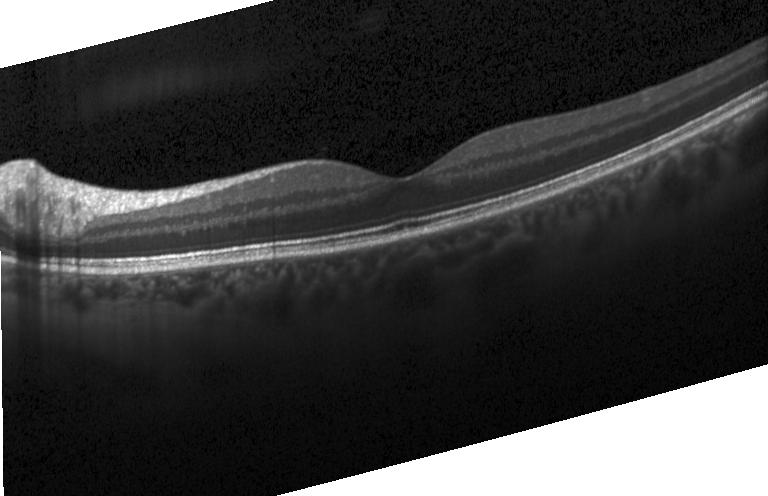

Dx: no evidence of choroidal neovascularization, diabetic macular edema, or drusen.